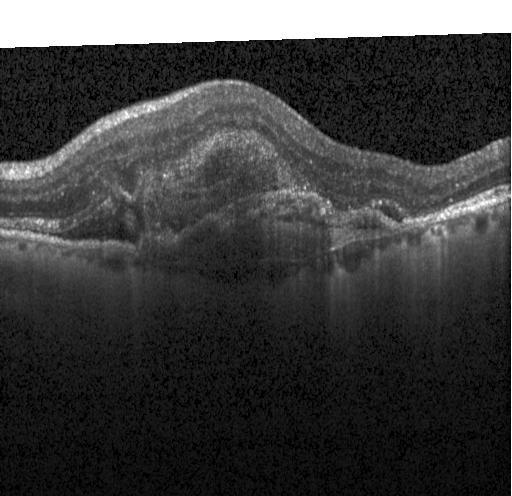 Centered on the fovea · OCT line scan
Impression: choroidal neovascularization.